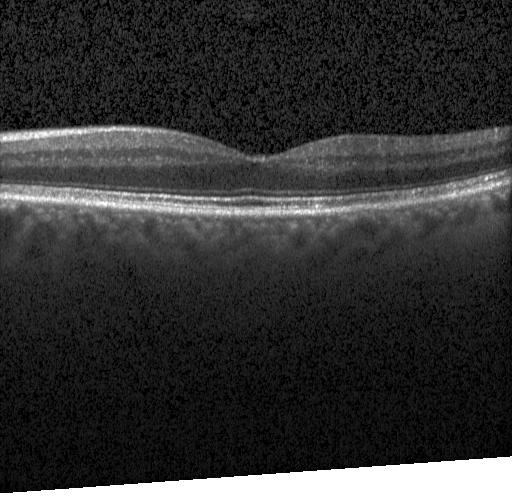 OCT line scan · Heidelberg Spectralis OCT system · through the macula · SD-OCT.
Assessment: neither CNV, DME, nor drusen.